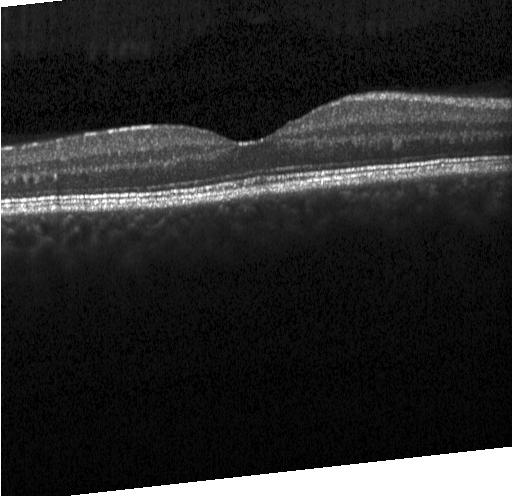

Macular OCT: neither CNV, DME, nor drusen.